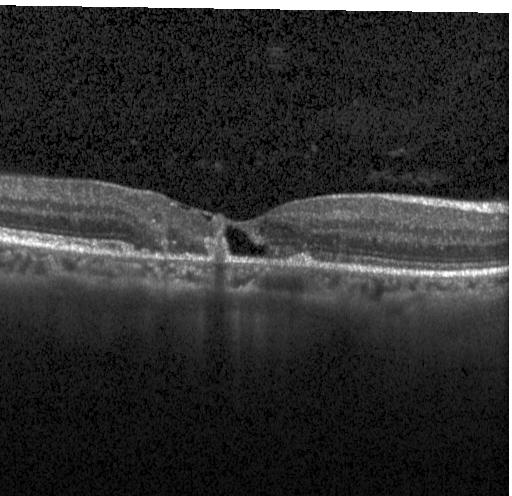
SD-OCT; horizontal scan through the fovea; Heidelberg Spectralis OCT system; optical coherence tomography scan — Impression: choroidal neovascularization.